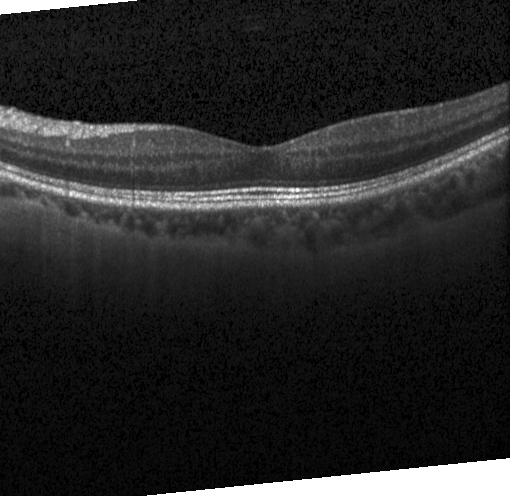
Macular OCT: no CNV, no DME, and no drusen.